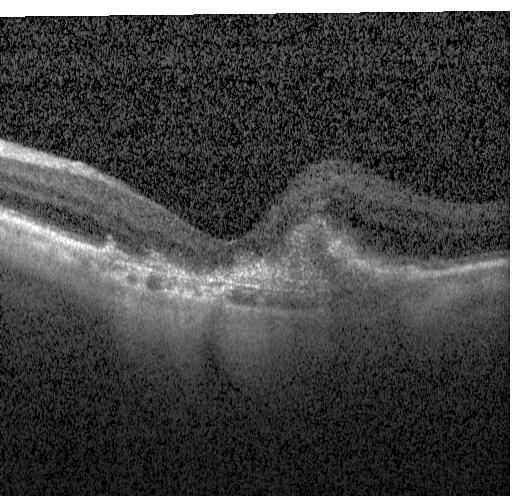

OCT finding: choroidal neovascularization (CNV).